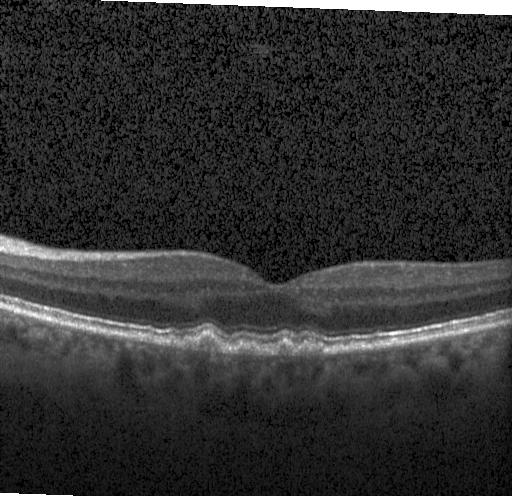

Finding: drusen.